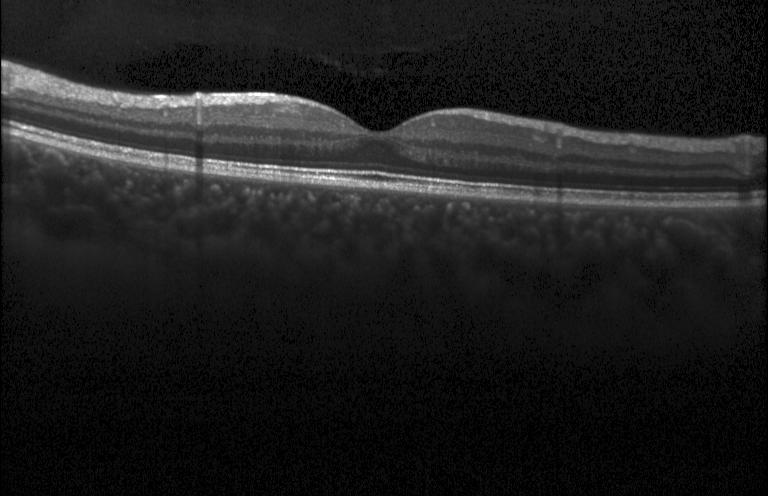 SD-OCT. Retinal OCT B-scan. Instrument: Heidelberg Spectralis
OCT finding: no evidence of choroidal neovascularization, diabetic macular edema, or drusen.